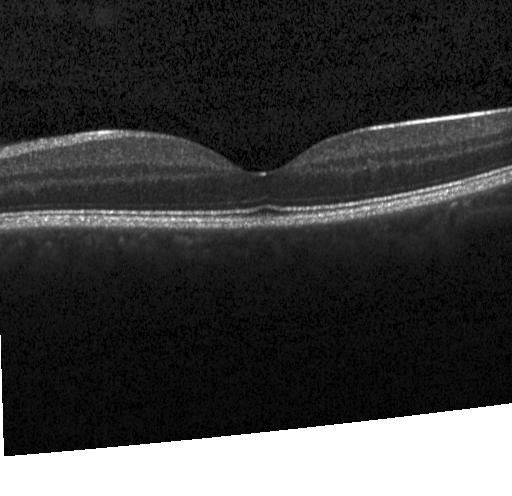

Optical coherence tomography scan, spectral-domain optical coherence tomography.
Impression: neither choroidal neovascularization, diabetic macular edema, nor drusen.